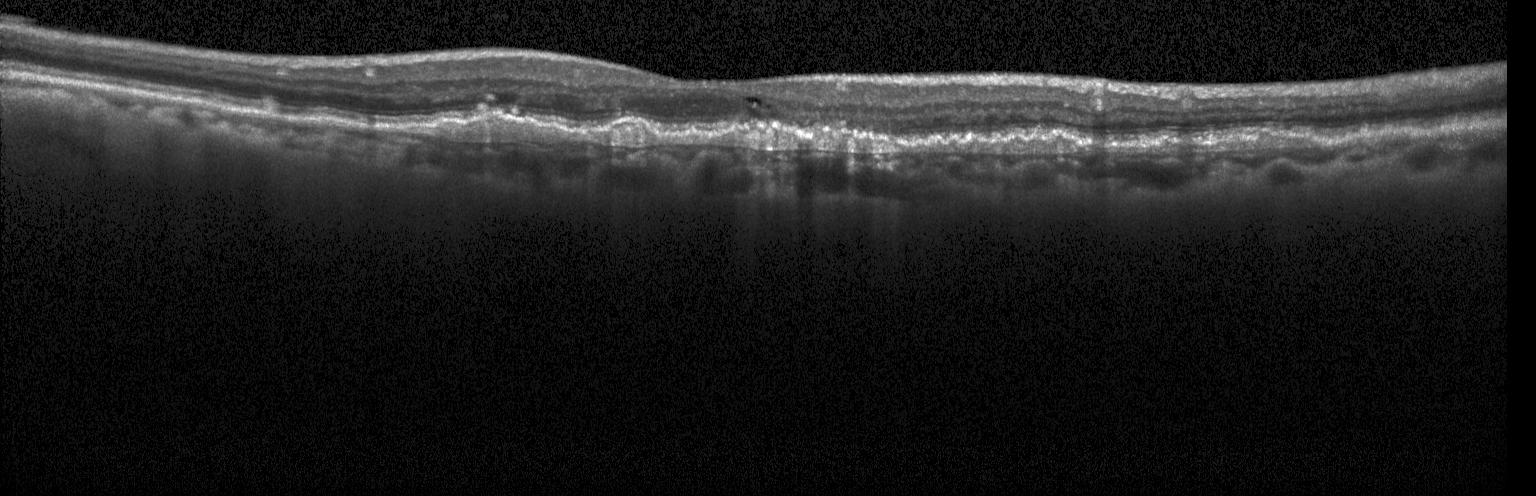
Macular OCT: CNV.